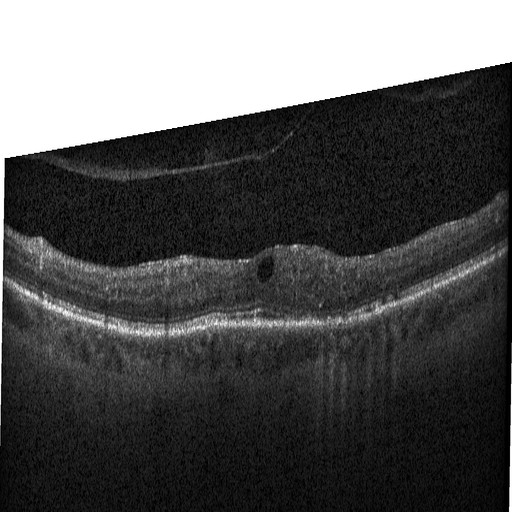

Impression: diabetic macular edema.